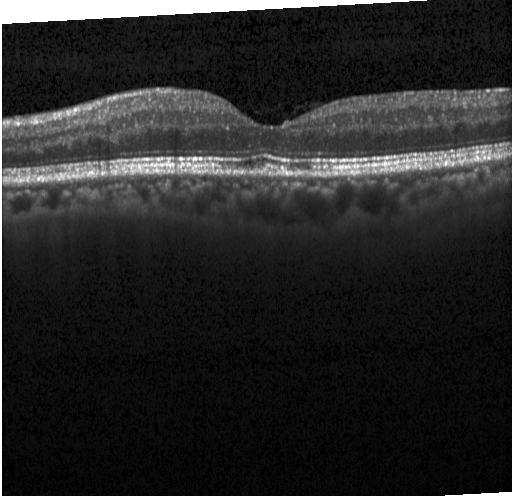 Horizontal scan through the fovea · Heidelberg Spectralis · OCT line scan · spectral-domain OCT
Diagnosis: neither CNV, DME, nor drusen.